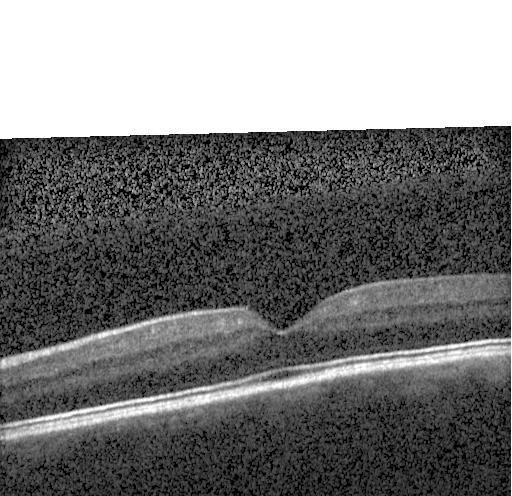
Acquired on a Heidelberg Spectralis · retinal OCT B-scan.
This B-scan demonstrates no choroidal neovascularization, diabetic macular edema, or drusen.